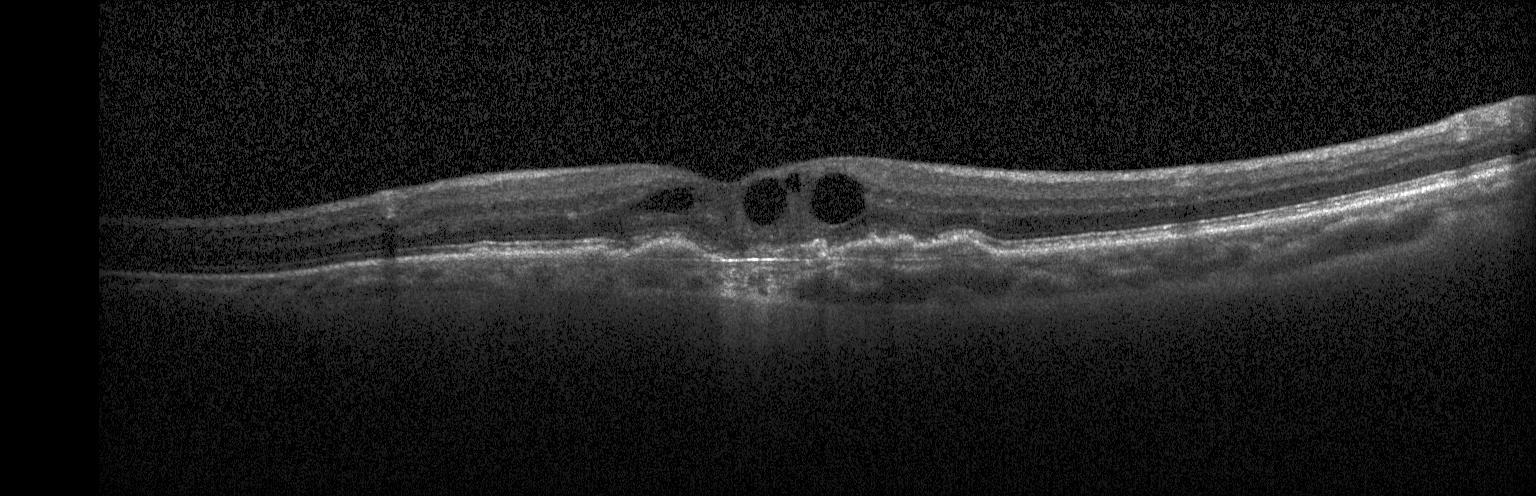 Dx: CNV.